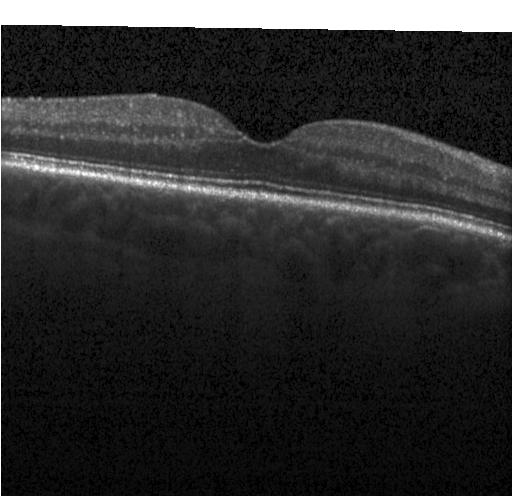
Impression: no choroidal neovascularization, diabetic macular edema, or drusen.